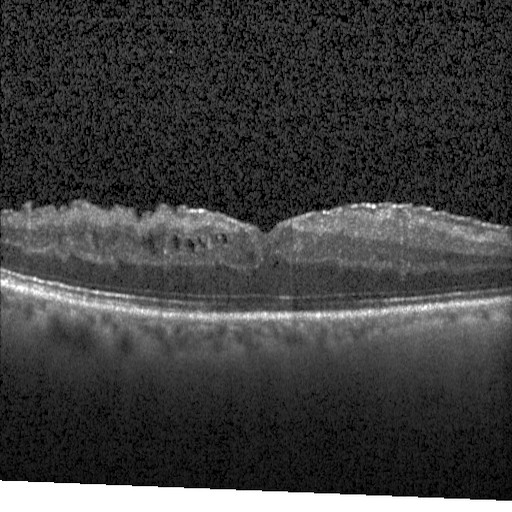 Fovea-centered, retinal OCT B-scan, acquired on a Heidelberg Spectralis — Macular OCT: diabetic macular edema.